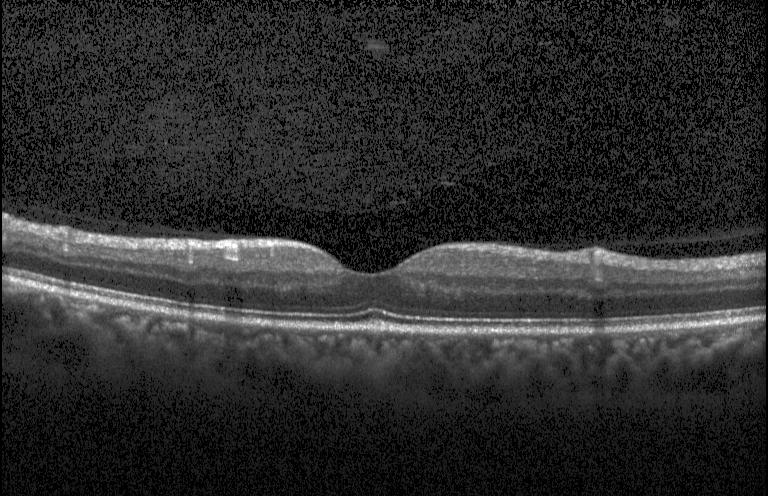 Finding: no choroidal neovascularization, no diabetic macular edema, and no drusen.